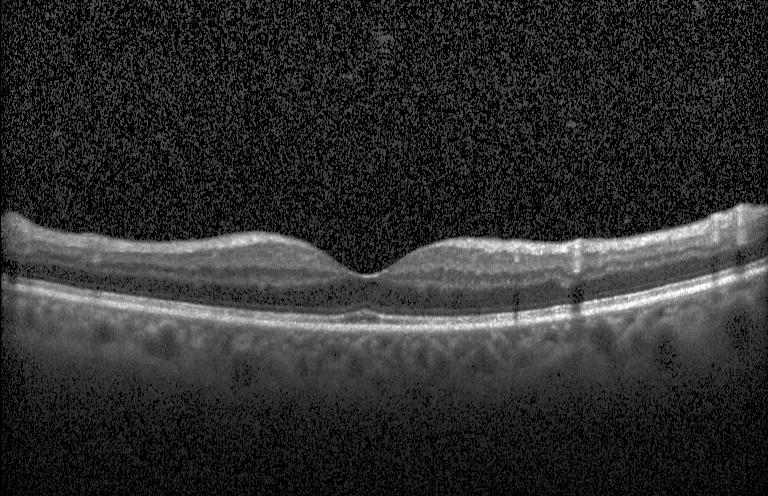

Impression: no choroidal neovascularization, diabetic macular edema, or drusen.